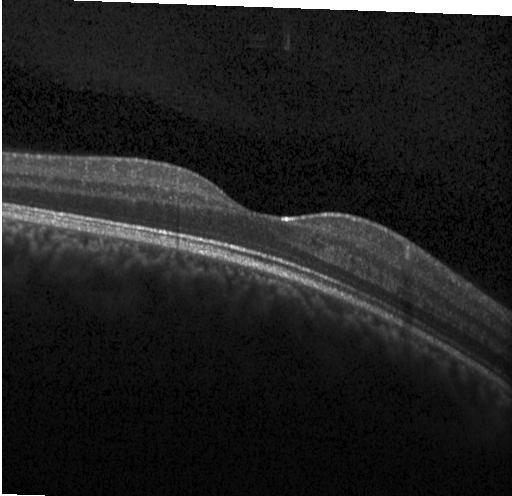
Retinal OCT B-scan, fovea-centered
Finding: no CNV, DME, or drusen.